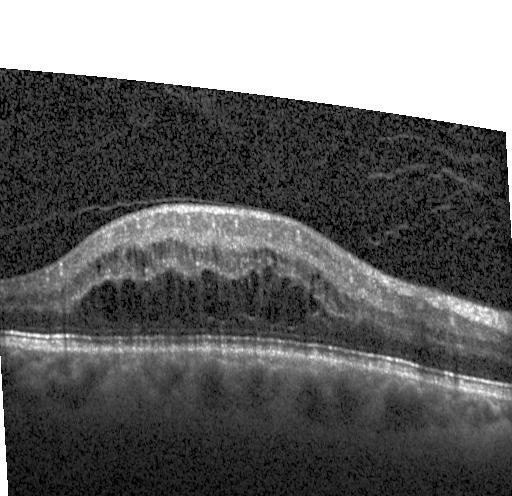 OCT B-scan.
The scan shows DME.